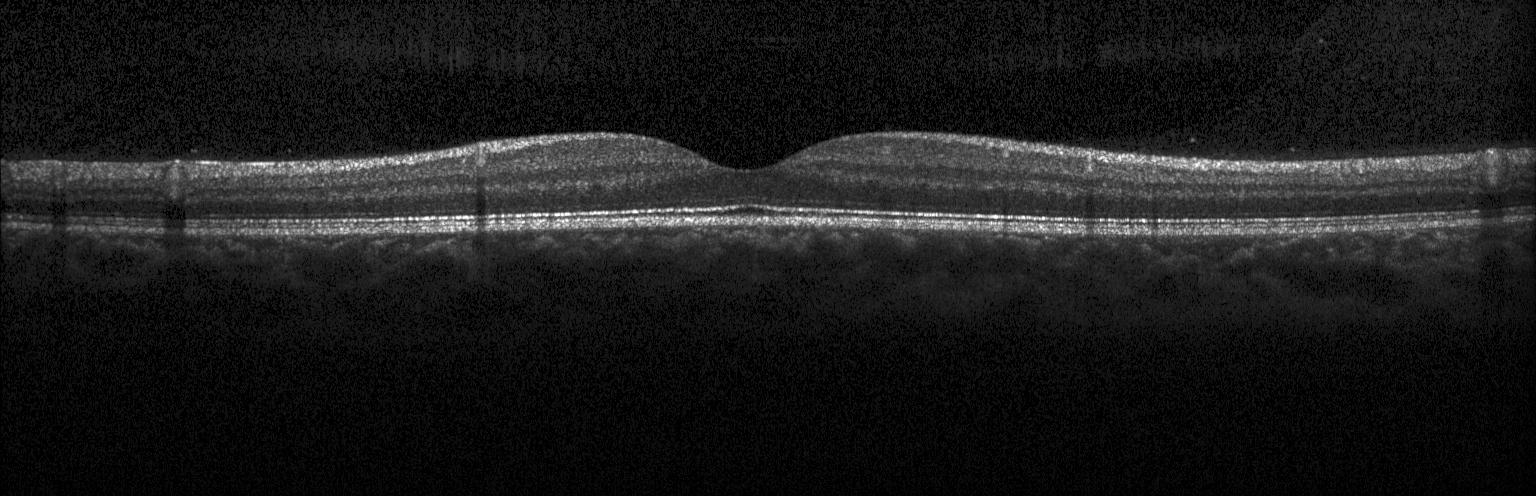
Impression: no evidence of choroidal neovascularization, diabetic macular edema, or drusen.